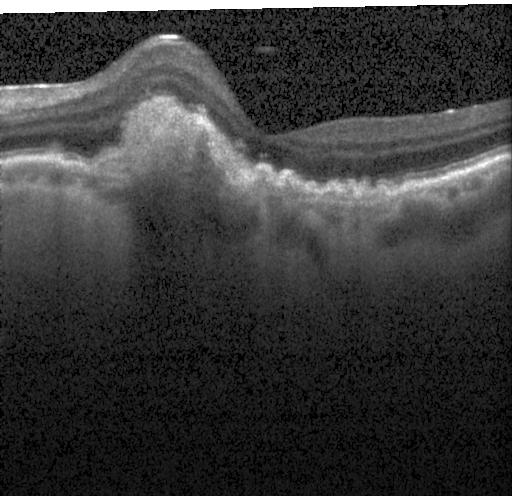
OCT scan showing a choroidal neovascular membrane.